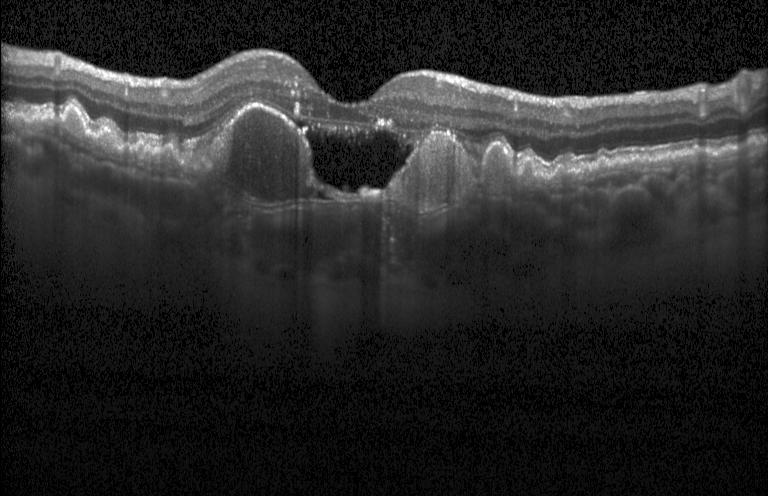
Impression: a choroidal neovascular membrane.